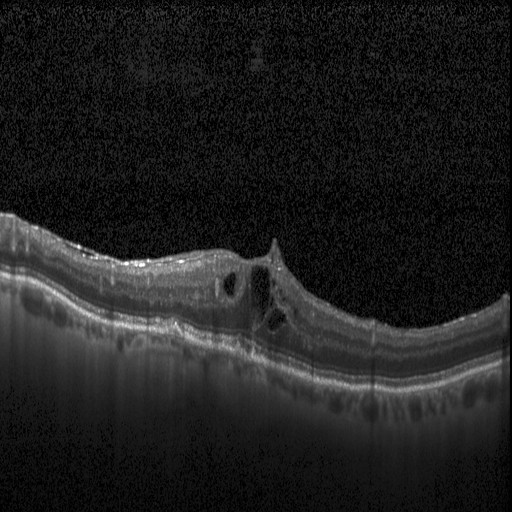 Optical coherence tomography B-scan
This B-scan demonstrates diabetic macular edema.